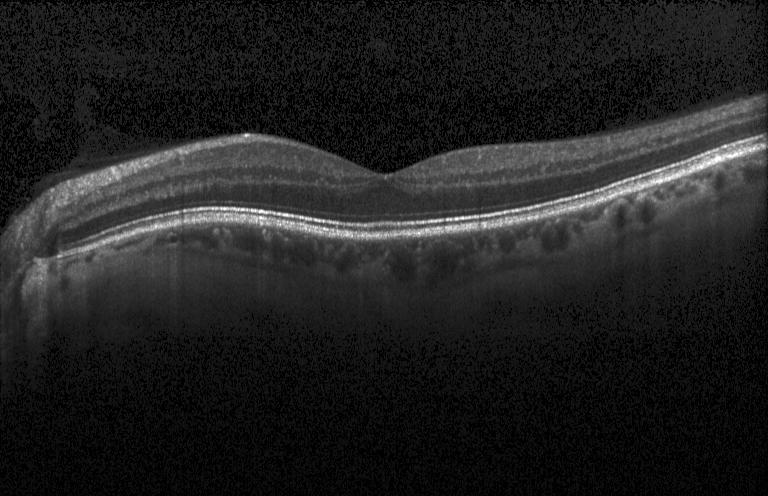
OCT scan showing no evidence of choroidal neovascularization, diabetic macular edema, or drusen.